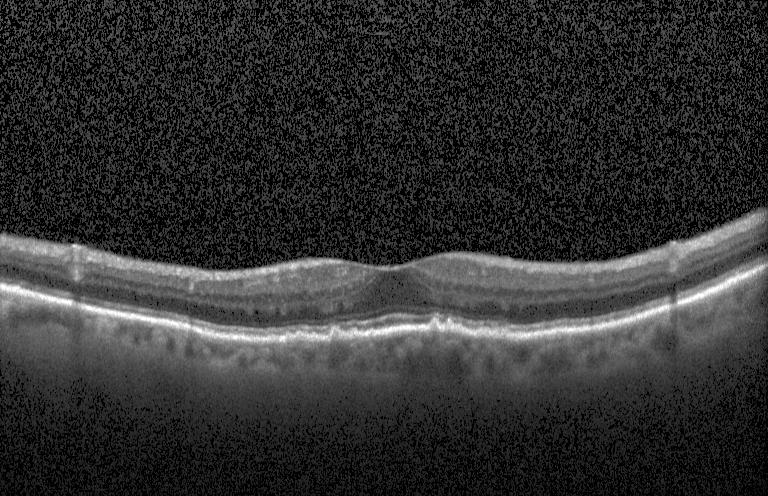

Diagnosis: multiple drusen.